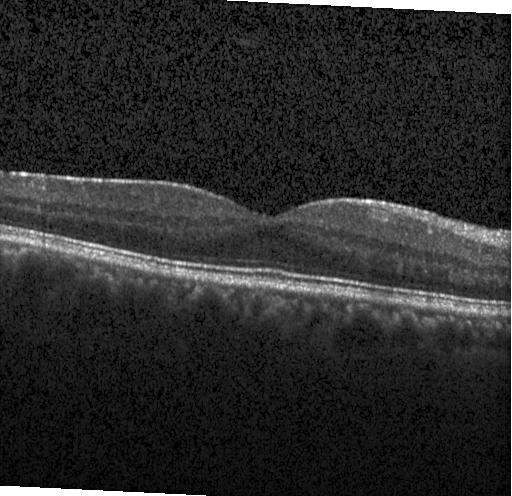 Macular scan · spectral-domain OCT · Heidelberg Spectralis · OCT line scan — OCT finding: no CNV, DME, or drusen.